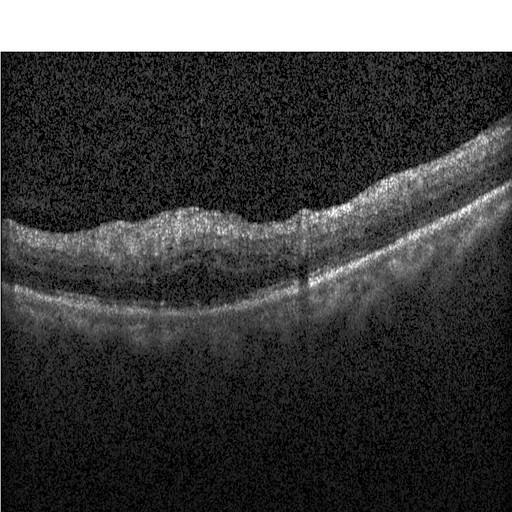
Optical coherence tomography scan; spectral-domain OCT; horizontal scan through the fovea; acquired on a Heidelberg Spectralis.
This B-scan demonstrates diabetic macular edema (DME).